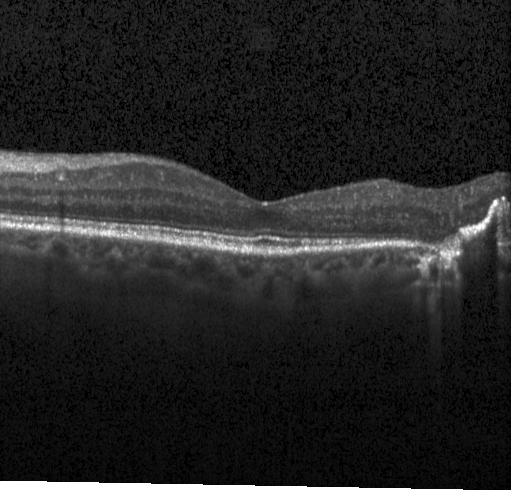 Macular scan, optical coherence tomography B-scan, spectral-domain optical coherence tomography, instrument: Heidelberg Spectralis — Impression: a choroidal neovascular membrane.